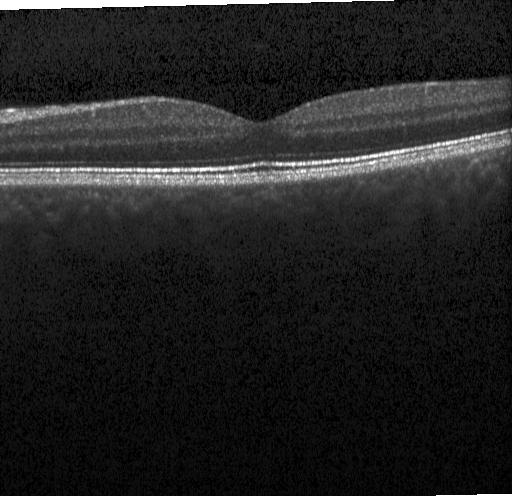 Finding: neither choroidal neovascularization, diabetic macular edema, nor drusen.